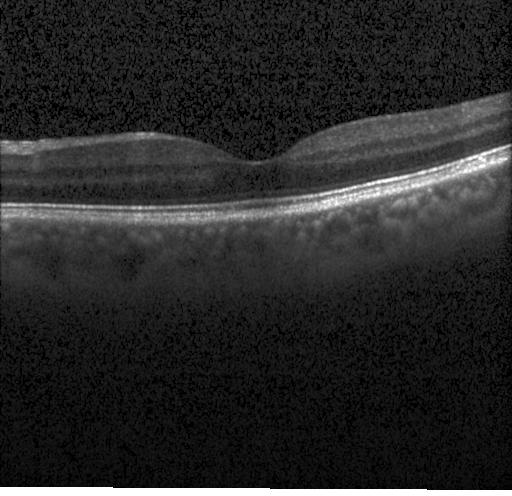

Optical coherence tomography scan · instrument: Heidelberg Spectralis
The scan shows no choroidal neovascularization, no diabetic macular edema, and no drusen.